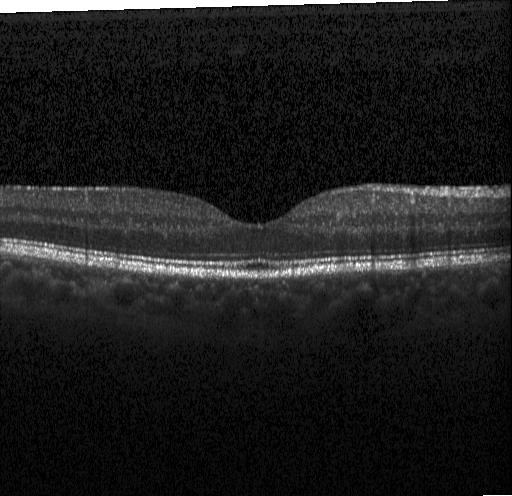
SD-OCT. Through the macula. Heidelberg Spectralis OCT system. Retinal OCT B-scan. OCT finding: no CNV, DME, or drusen.